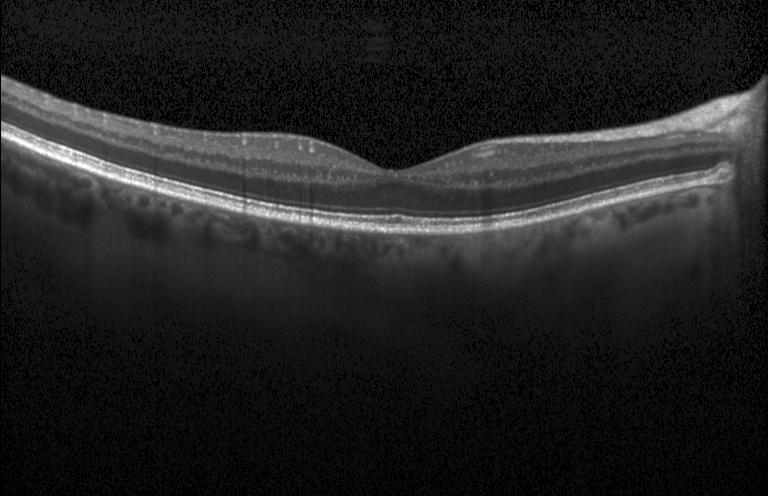

Macular scan · SD-OCT · optical coherence tomography B-scan · Heidelberg Spectralis OCT system
The scan shows neither choroidal neovascularization, diabetic macular edema, nor drusen.